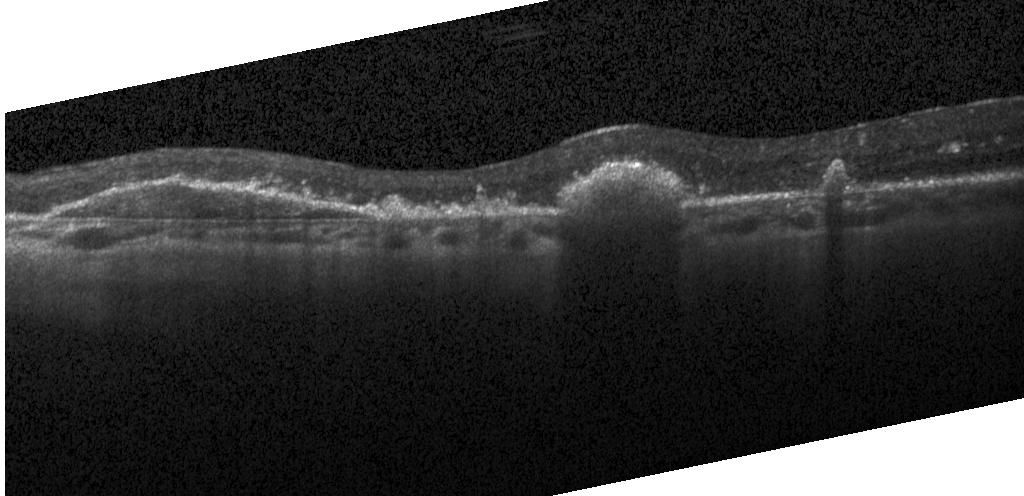
Horizontal scan through the fovea · acquired on a Heidelberg Spectralis · SD-OCT · optical coherence tomography B-scan. Macular OCT: a choroidal neovascular membrane.